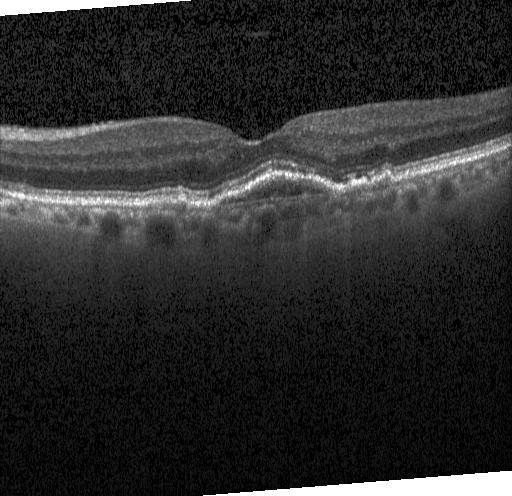 Optical coherence tomography scan. Through the macula. Instrument: Heidelberg Spectralis. Spectral-domain optical coherence tomography. Dx: choroidal neovascularization (CNV).